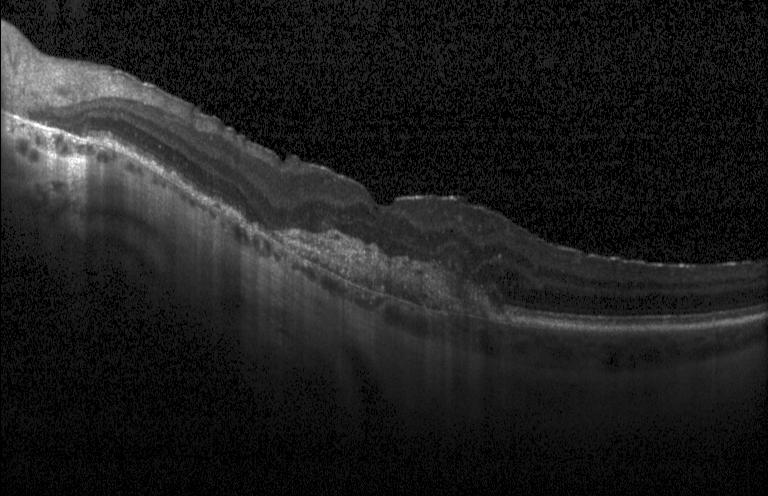

Acquired on a Heidelberg Spectralis. Through the macula. OCT B-scan
Diagnosis: CNV.